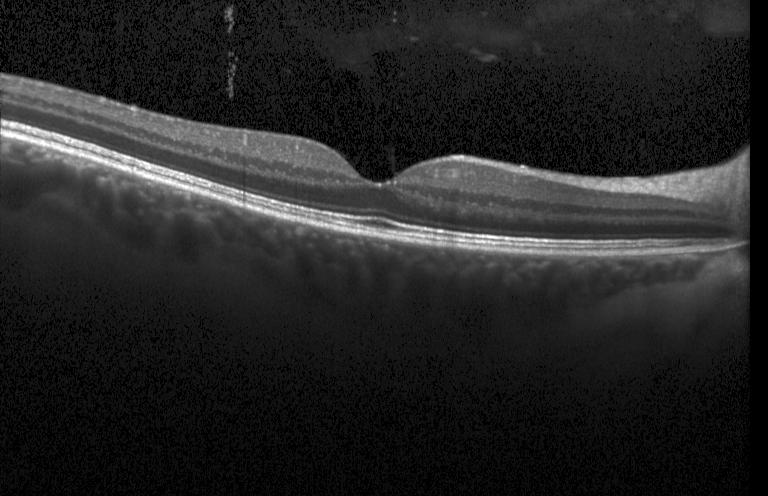 OCT line scan; through the macula; Heidelberg Spectralis; SD-OCT.
This B-scan demonstrates neither choroidal neovascularization, diabetic macular edema, nor drusen.